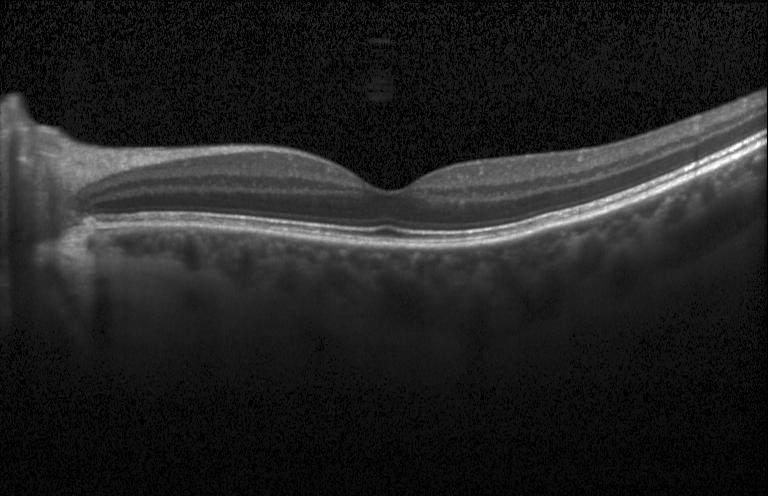

OCT B-scan.
Impression: no choroidal neovascularization, no diabetic macular edema, and no drusen.